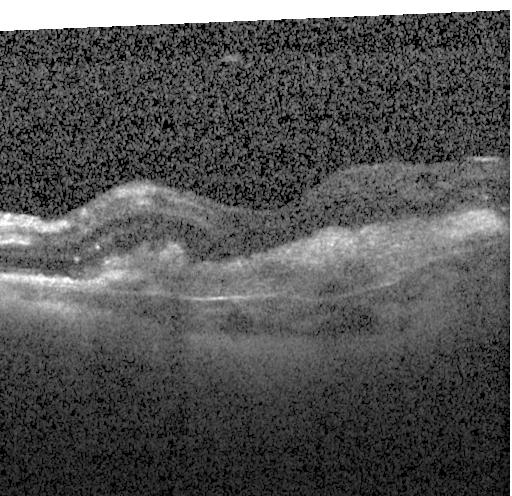
Retinal OCT B-scan
Macular OCT: CNV.